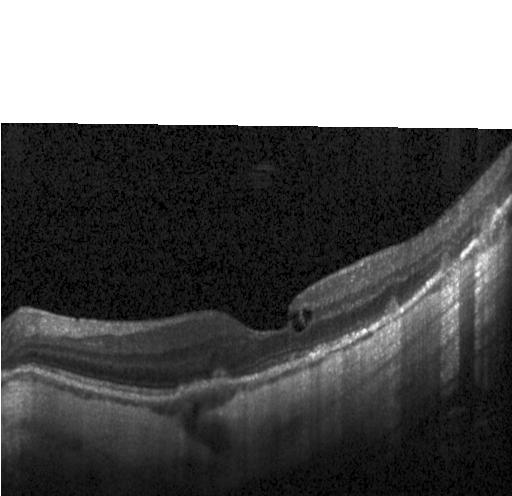

Retinal OCT B-scan
The scan shows a choroidal neovascular membrane.